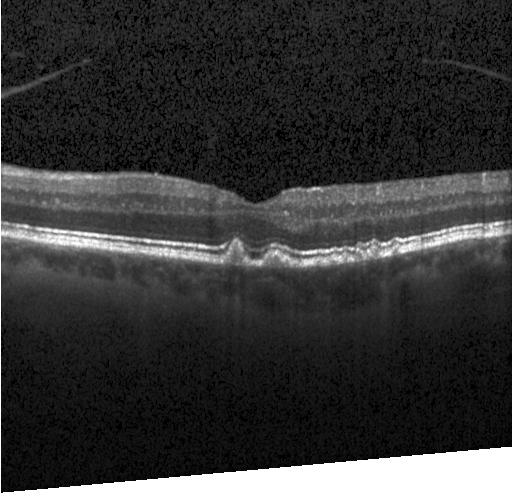
Retinal OCT B-scan
Diagnosis: multiple drusen.